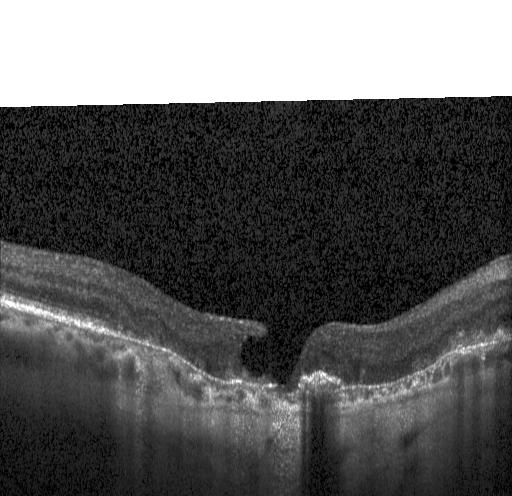 Spectral-domain optical coherence tomography · through the macula · optical coherence tomography B-scan — Diagnosis: CNV.